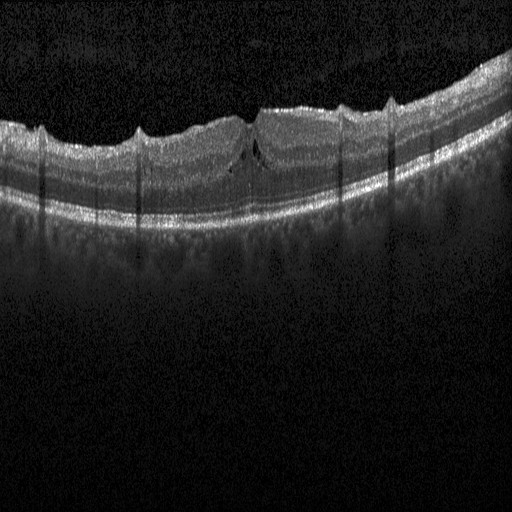 Impression: diabetic macular edema.